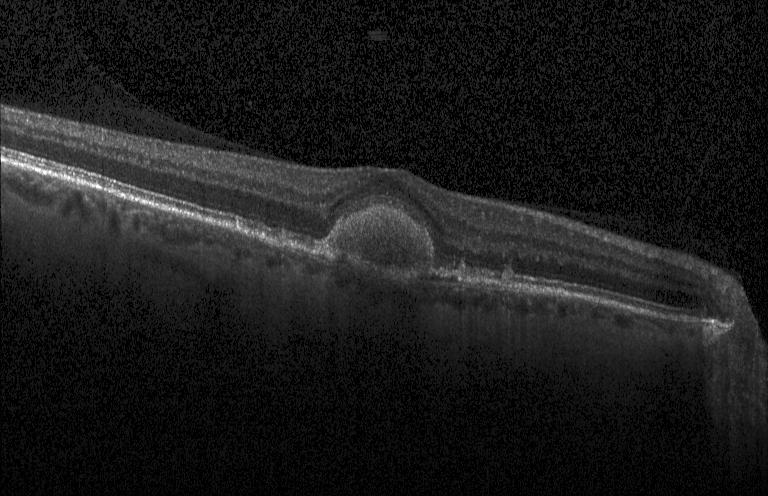 Impression: a choroidal neovascular membrane.